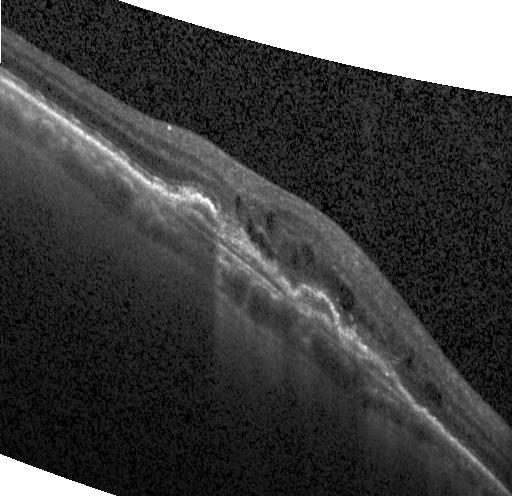

Through the macula, retinal OCT cross-section, SD-OCT, Heidelberg Spectralis OCT system.
Diagnosis: a choroidal neovascular membrane.